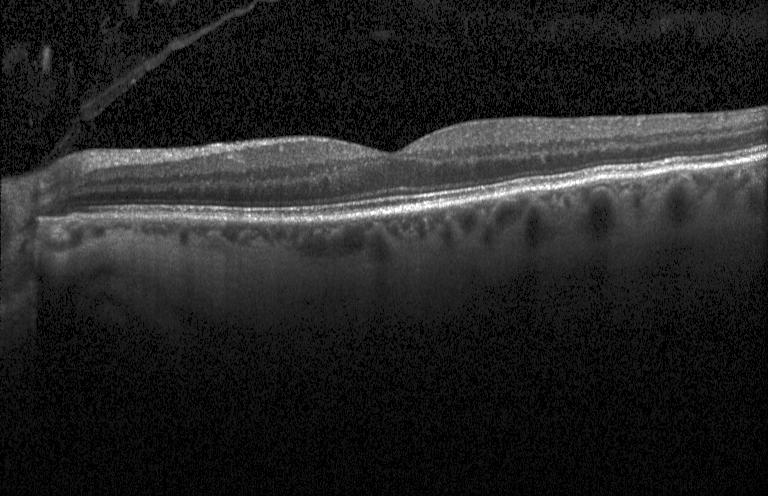 OCT B-scan — Dx: no choroidal neovascularization, diabetic macular edema, or drusen.